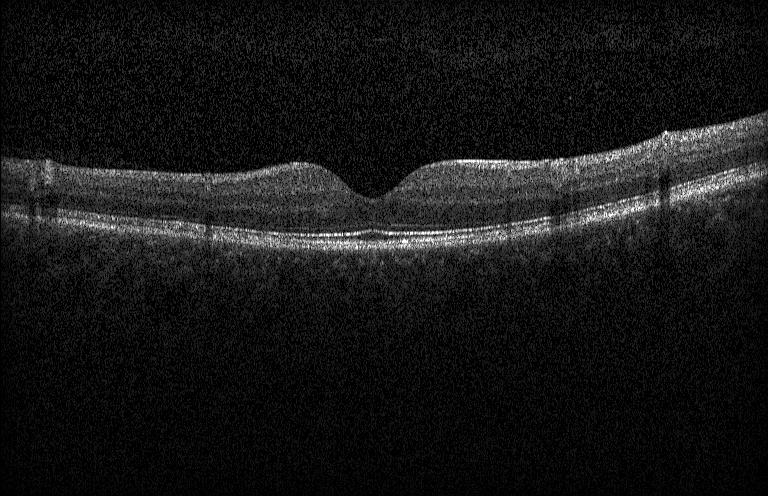
SD-OCT. Acquired on a Heidelberg Spectralis. OCT line scan — This B-scan demonstrates no evidence of choroidal neovascularization, diabetic macular edema, or drusen.